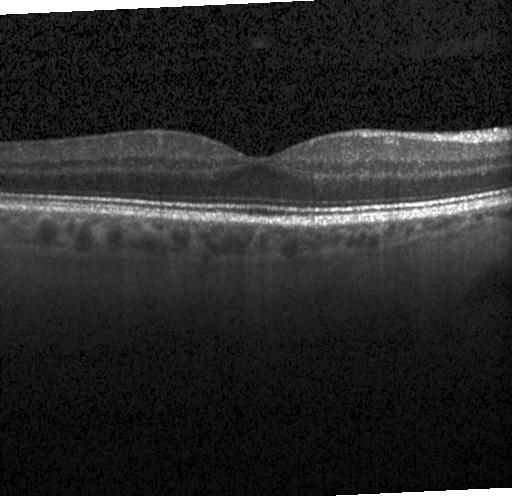

Retinal OCT B-scan · Heidelberg Spectralis OCT system.
Finding: neither choroidal neovascularization, diabetic macular edema, nor drusen.